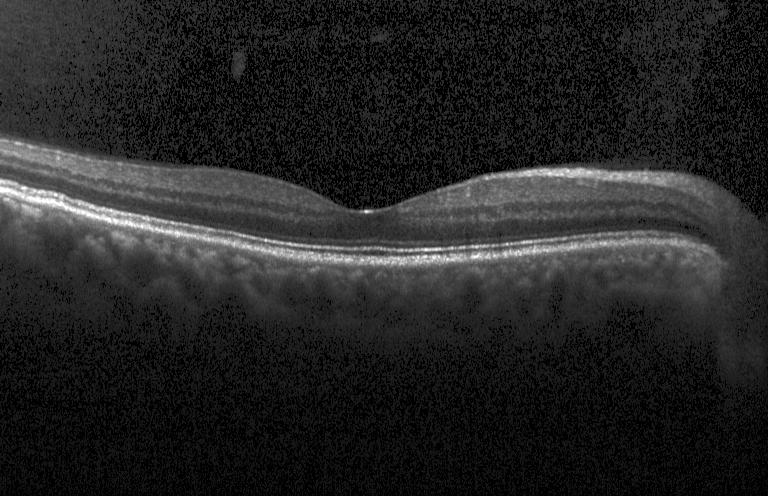
This B-scan demonstrates no choroidal neovascularization, no diabetic macular edema, and no drusen.